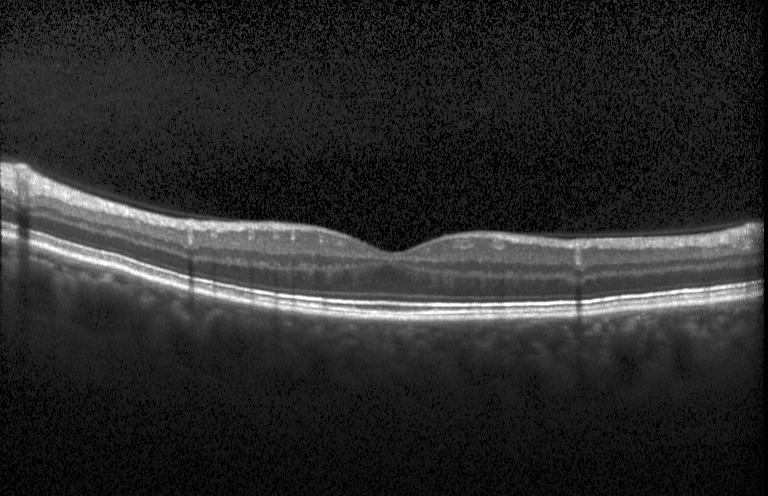

Macular scan, optical coherence tomography scan, Heidelberg Spectralis. The scan shows no CNV, DME, or drusen.